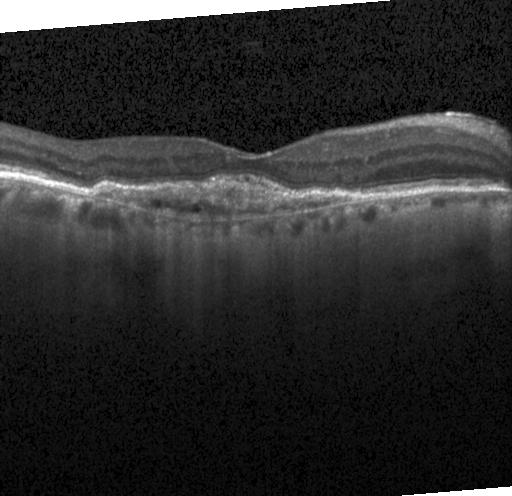 Diagnosis: CNV.